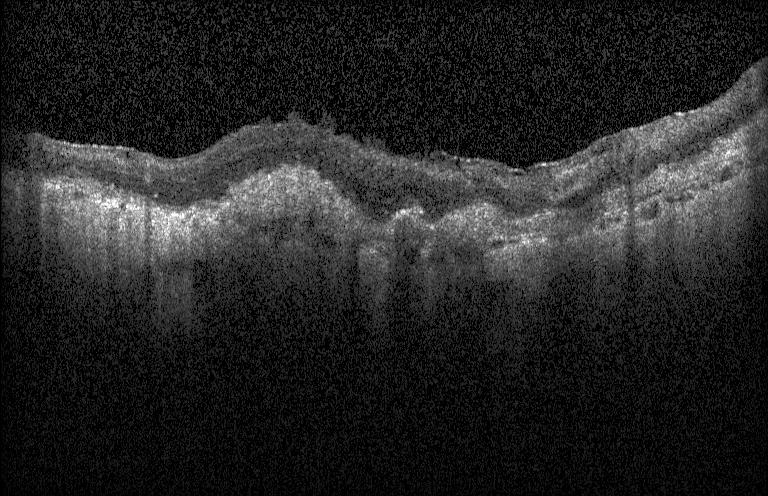
Heidelberg Spectralis, SD-OCT, horizontal scan through the fovea, optical coherence tomography scan
Finding: CNV.